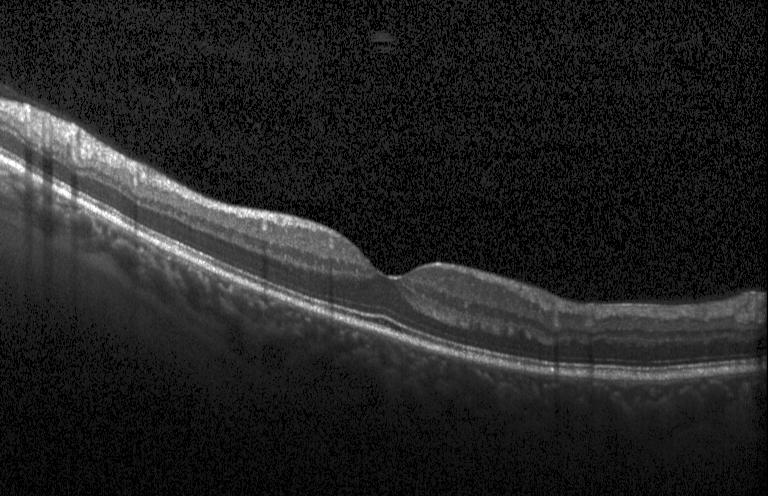

Macular scan · retinal OCT cross-section · Heidelberg Spectralis OCT system · spectral-domain OCT — Macular OCT: neither choroidal neovascularization, diabetic macular edema, nor drusen.